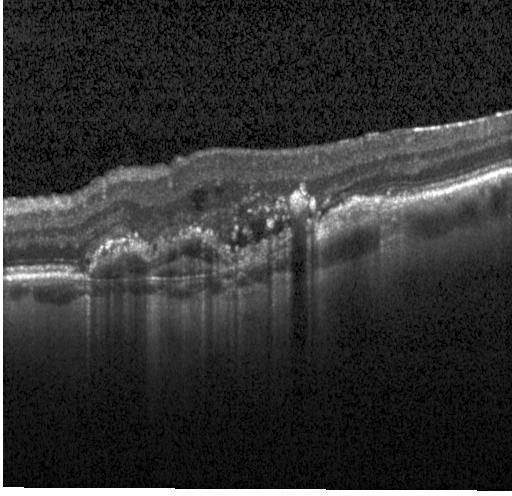 Dx: a choroidal neovascular membrane.